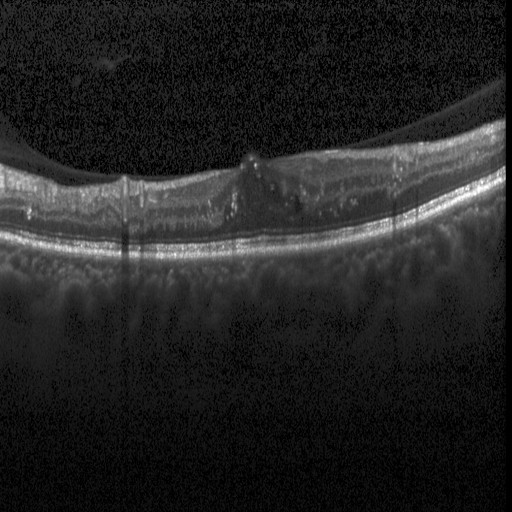 OCT line scan.
OCT finding: diabetic macular edema (DME).